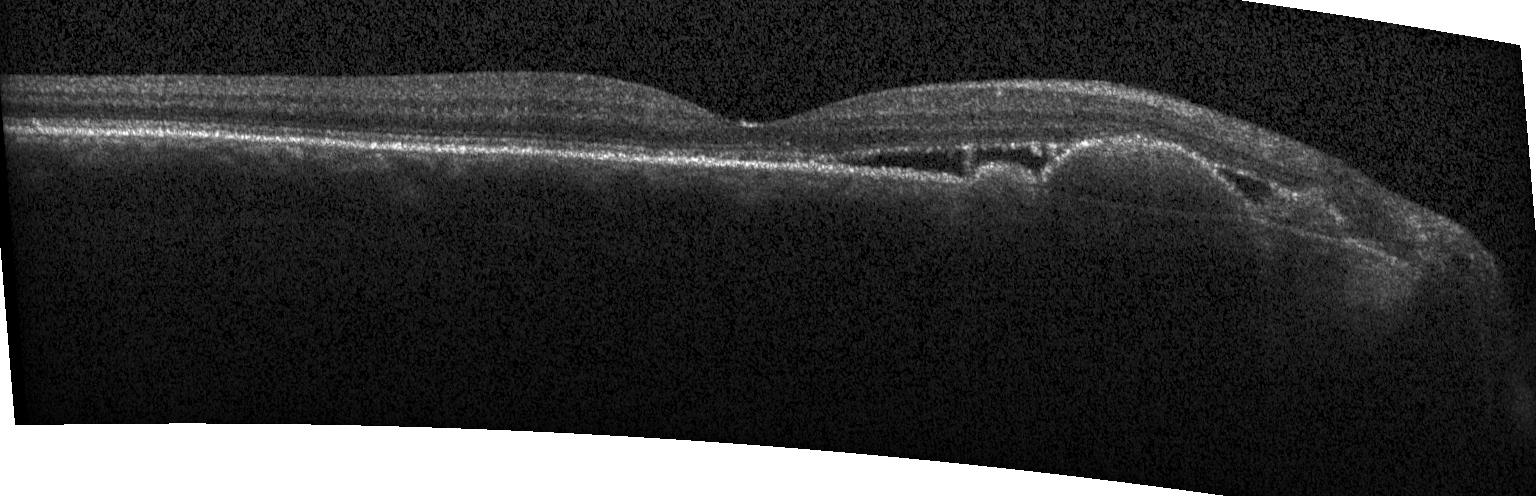
Diagnosis: a choroidal neovascular membrane.